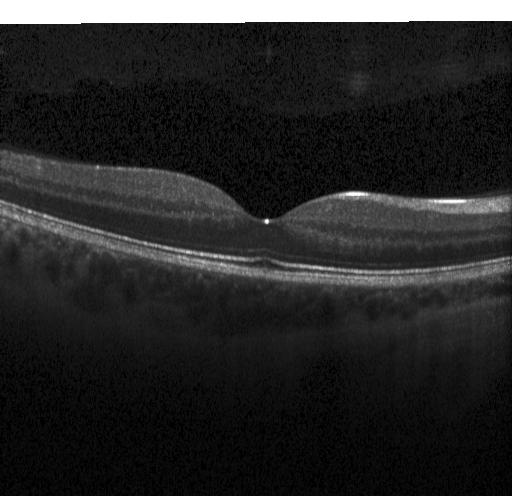
SD-OCT; optical coherence tomography B-scan.
Impression: no choroidal neovascularization, diabetic macular edema, or drusen.